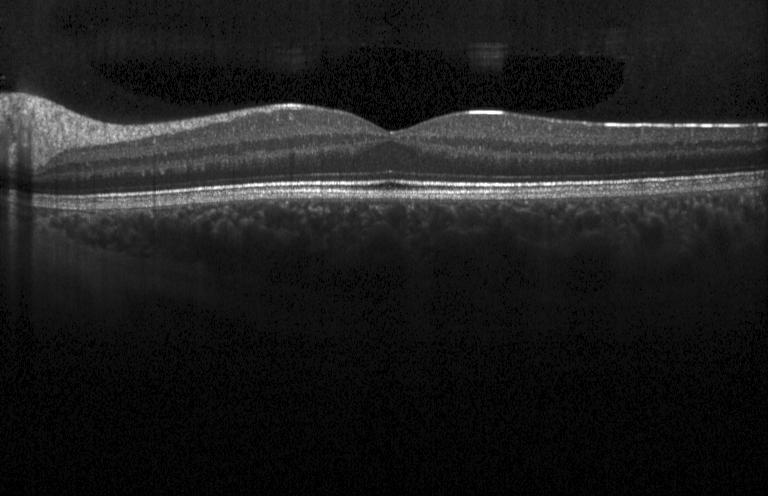

Finding: no evidence of CNV, DME, or drusen.